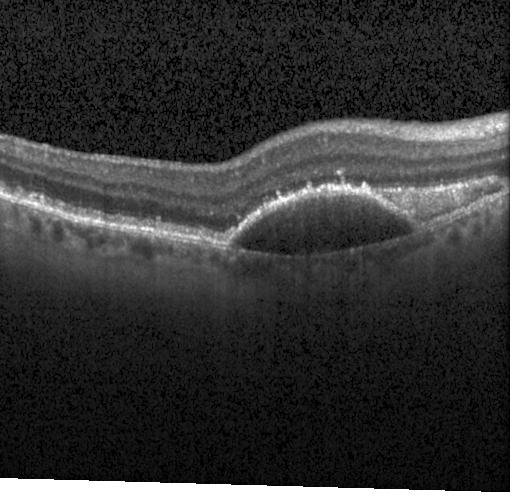 OCT scan showing a choroidal neovascular membrane.